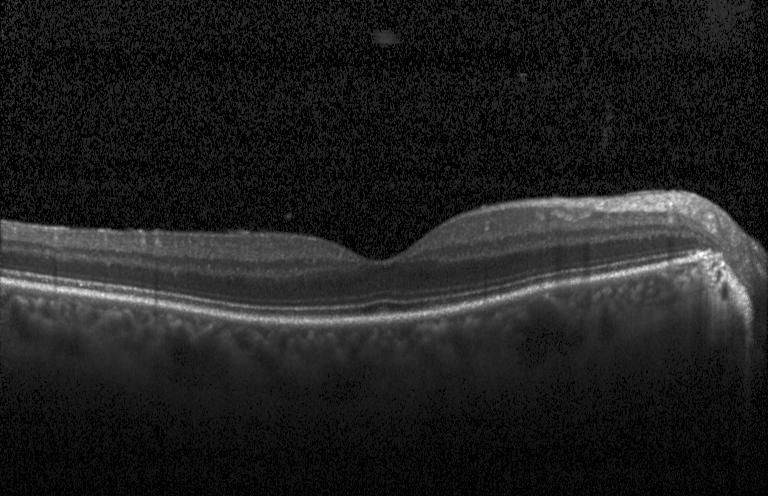 Dx: neither CNV, DME, nor drusen.